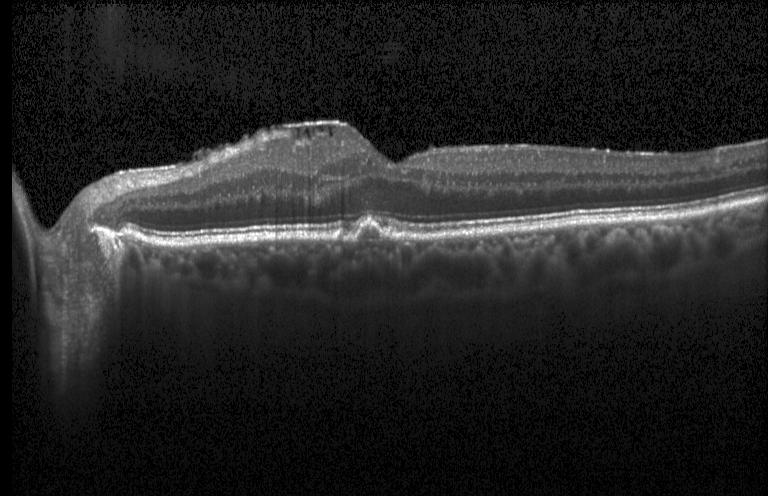 Optical coherence tomography B-scan. This B-scan demonstrates sub-RPE drusenoid deposits.